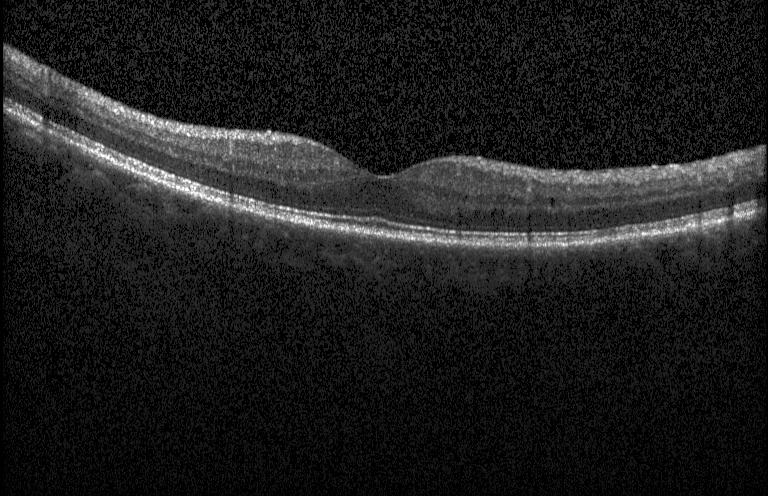 Retinal OCT B-scan. Impression: no choroidal neovascularization, diabetic macular edema, or drusen.